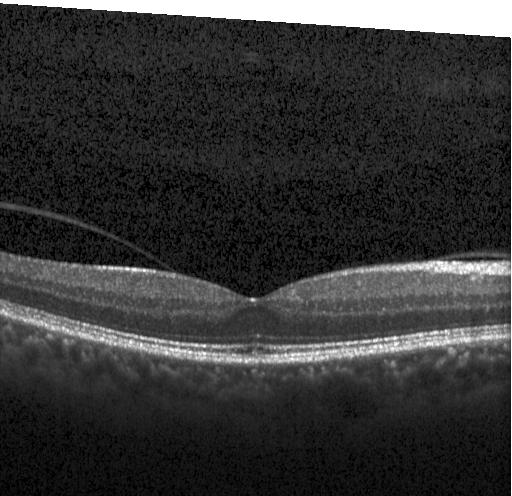
Optical coherence tomography scan · Heidelberg Spectralis. Finding: no evidence of CNV, DME, or drusen.